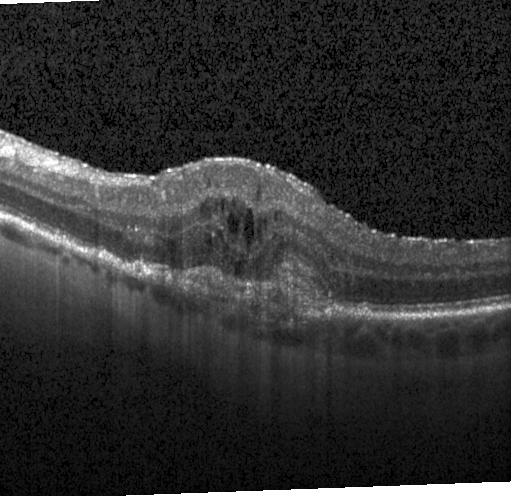

Macular scan · retinal OCT cross-section · Heidelberg Spectralis
Impression: CNV.